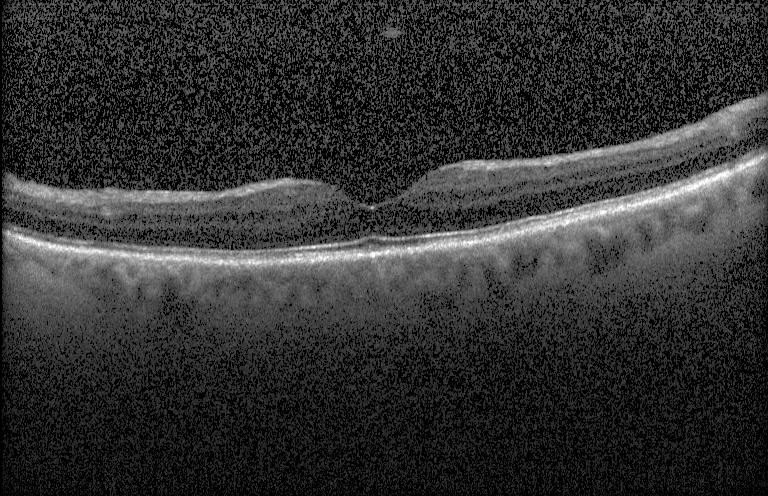
Spectral-domain OCT B-scan: no evidence of CNV, DME, or drusen.